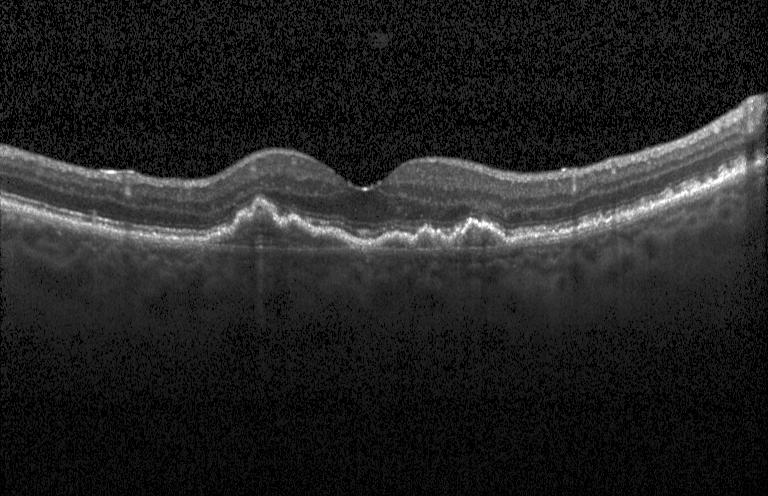

Fovea-centered. OCT B-scan. This B-scan demonstrates a choroidal neovascular membrane.